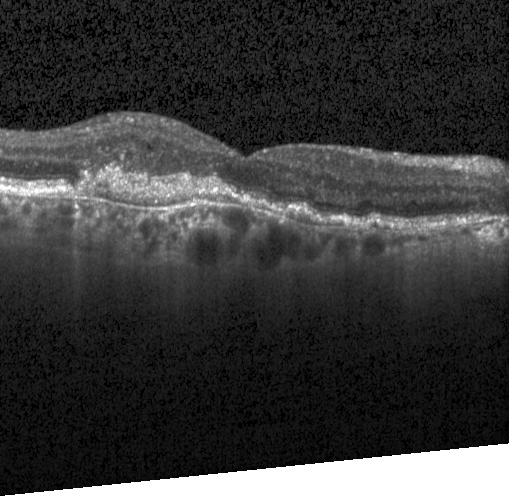
Optical coherence tomography scan, instrument: Heidelberg Spectralis — A choroidal neovascular membrane.